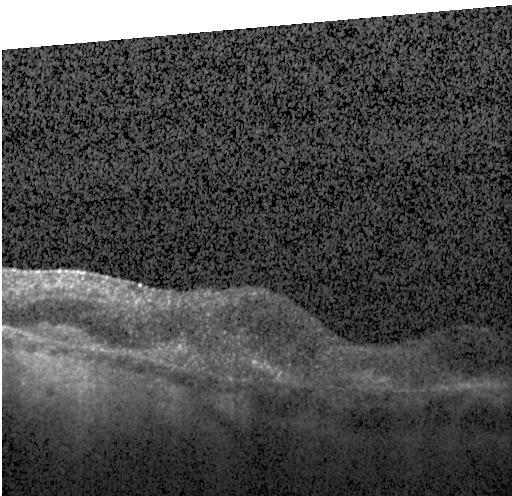
Spectral-domain optical coherence tomography; horizontal scan through the fovea; OCT line scan; Heidelberg Spectralis — The scan shows a choroidal neovascular membrane.